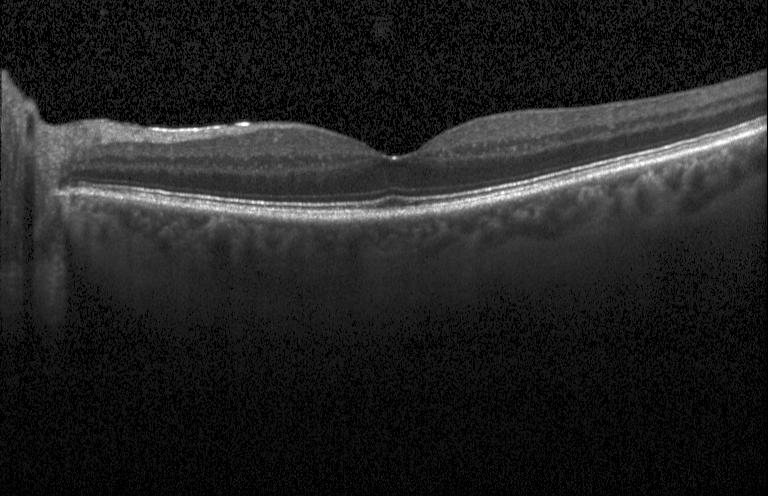
Finding: no CNV, DME, or drusen.